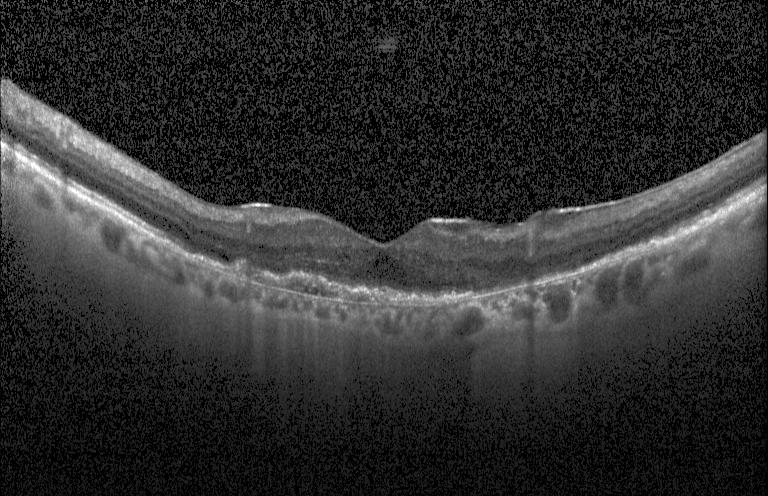
Optical coherence tomography scan. Heidelberg Spectralis OCT system. Diagnosis: choroidal neovascularization (CNV).